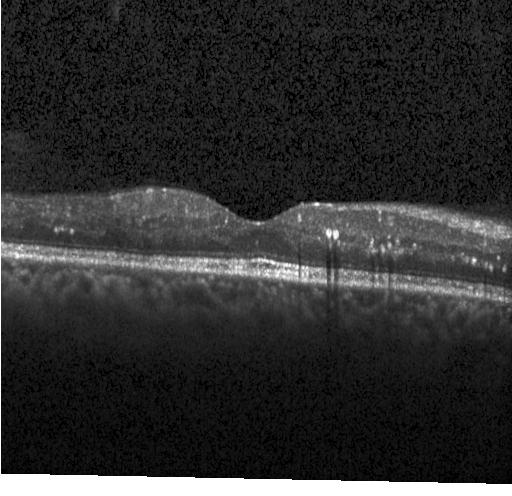

Optical coherence tomography scan; spectral-domain OCT; instrument: Heidelberg Spectralis
Diabetic macular edema.